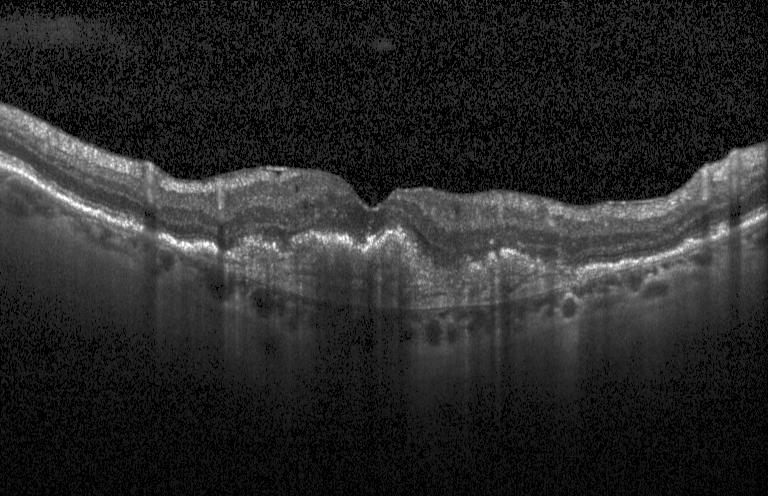
Centered on the fovea, SD-OCT, acquired on a Heidelberg Spectralis, optical coherence tomography scan. Finding: choroidal neovascularization.